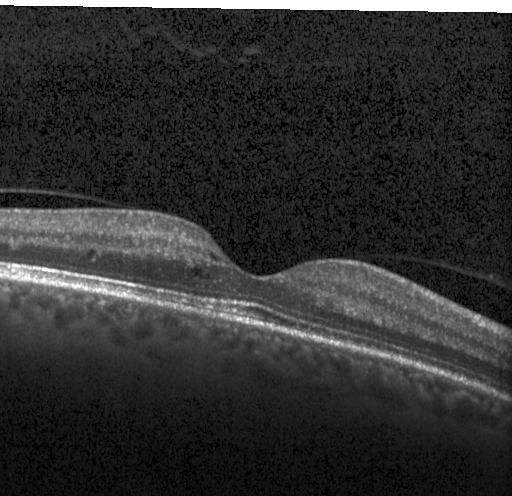
Spectral-domain OCT, instrument: Heidelberg Spectralis, retinal OCT cross-section.
Dx: diabetic macular edema.